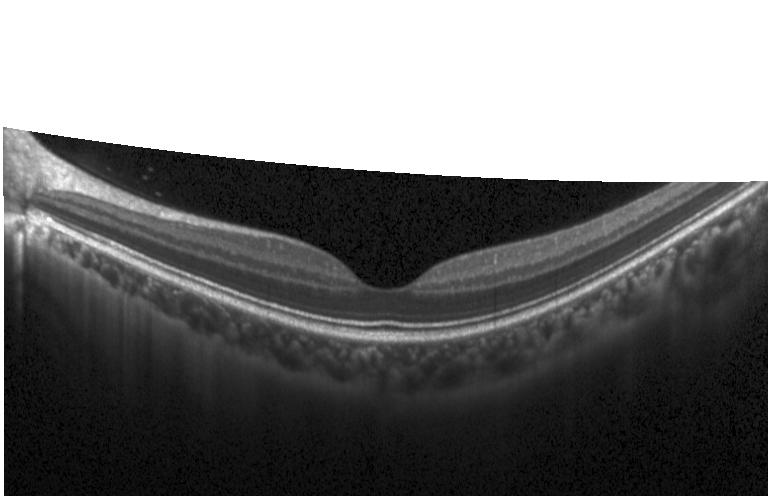 Spectral-domain OCT B-scan: no evidence of CNV, DME, or drusen.